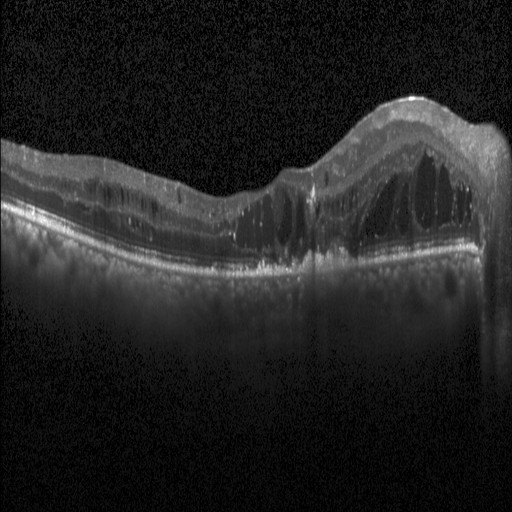 Impression: diabetic macular edema.